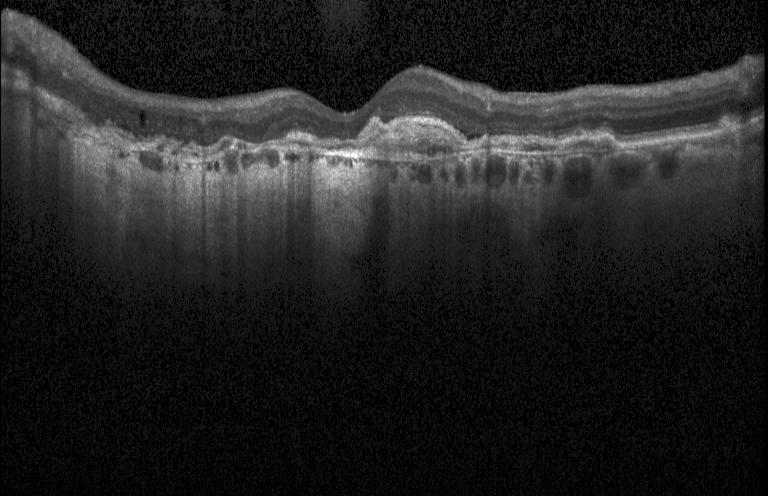
Retinal OCT cross-section — Impression: CNV.